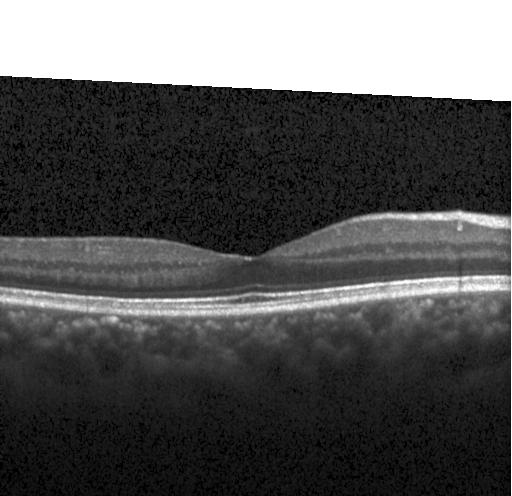
Retinal OCT cross-section
Macular OCT: no CNV, no DME, and no drusen.